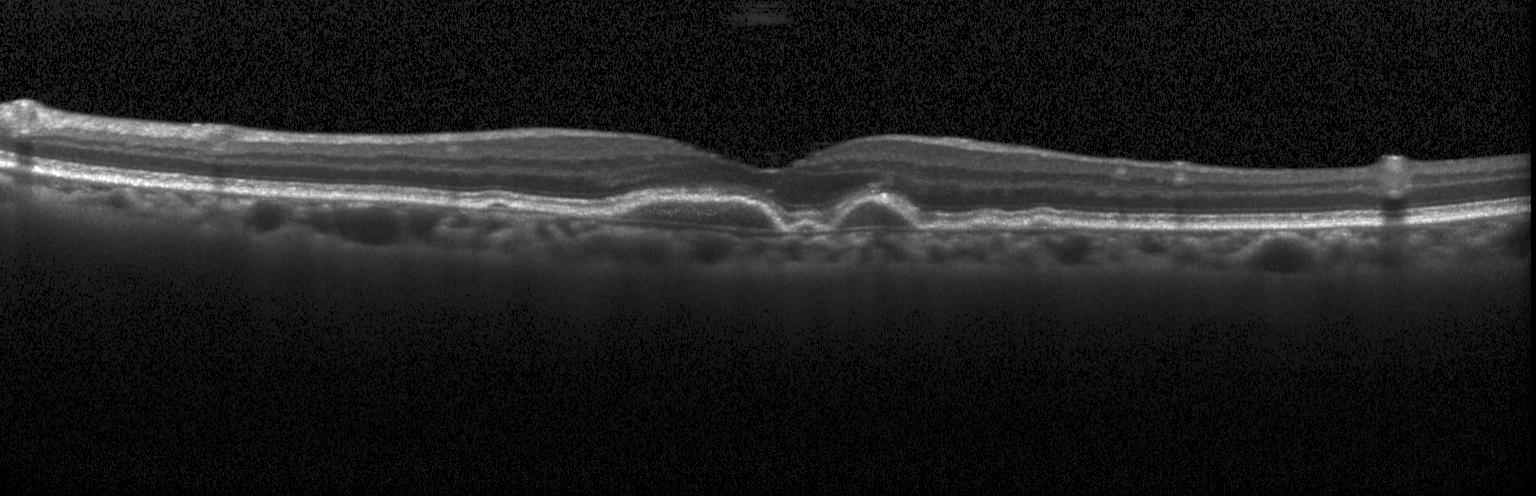

Retinal OCT B-scan. Macular scan. Heidelberg Spectralis OCT system
This B-scan demonstrates choroidal neovascularization.